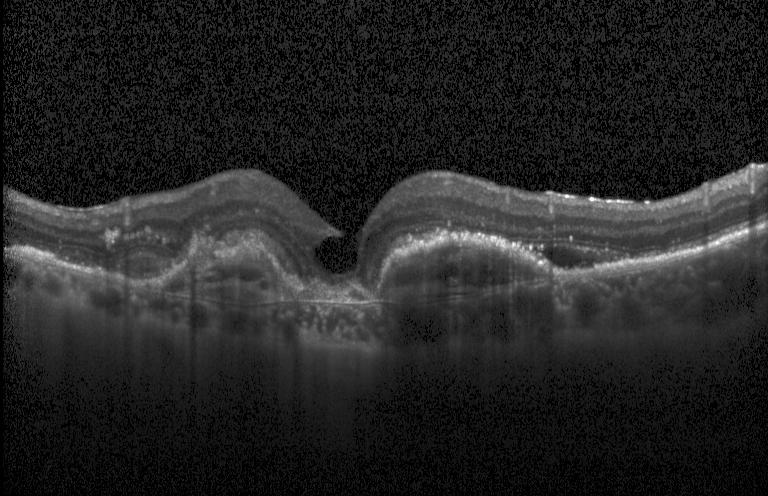 Impression: a choroidal neovascular membrane.